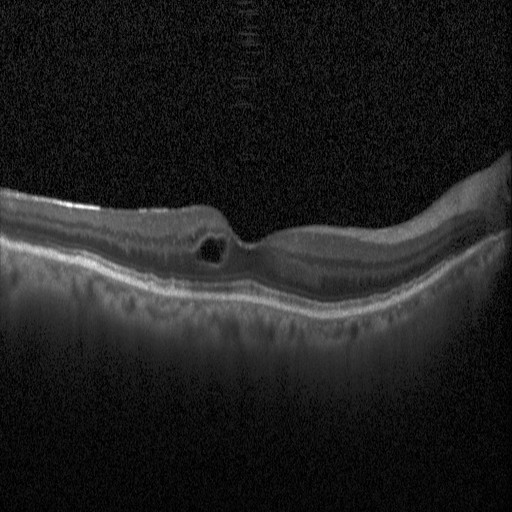
OCT B-scan
Impression: diabetic macular edema.